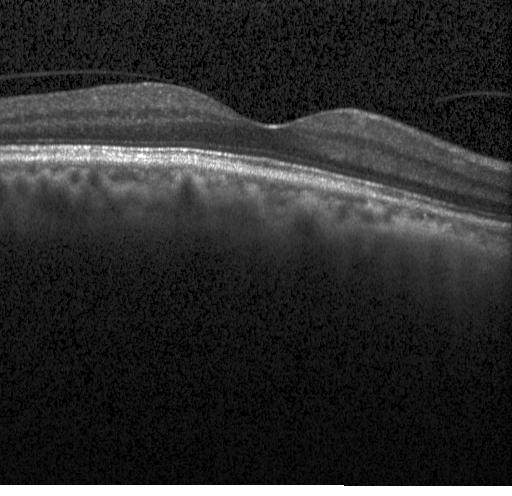
SD-OCT. Optical coherence tomography scan
This B-scan demonstrates neither choroidal neovascularization, diabetic macular edema, nor drusen.